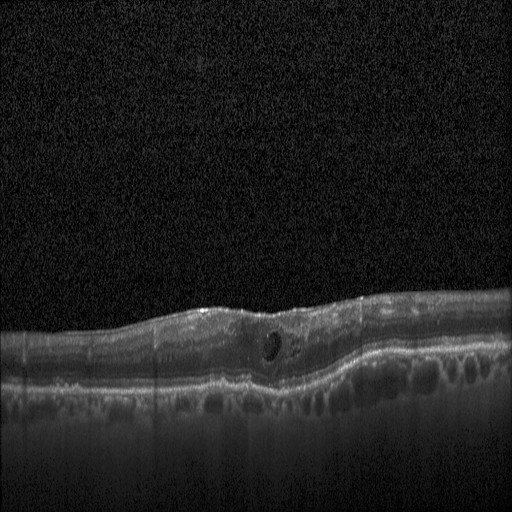
Dx: DME.